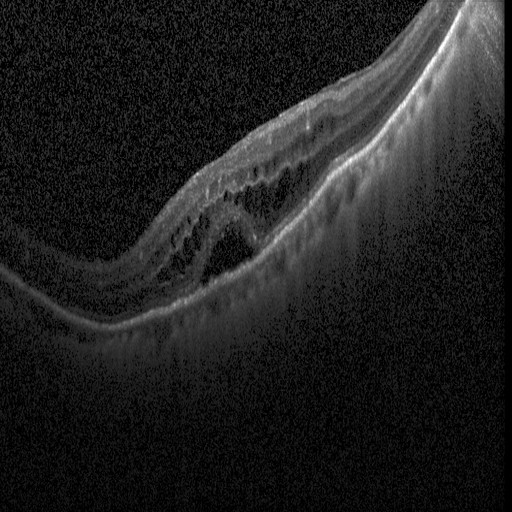

Optical coherence tomography scan, through the macula, Heidelberg Spectralis OCT system — Impression: diabetic macular edema (DME).